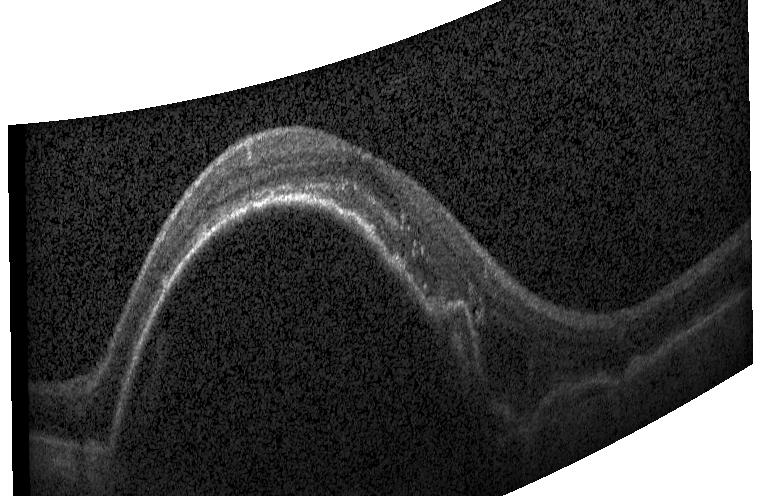 Optical coherence tomography B-scan. Macular OCT: a choroidal neovascular membrane.